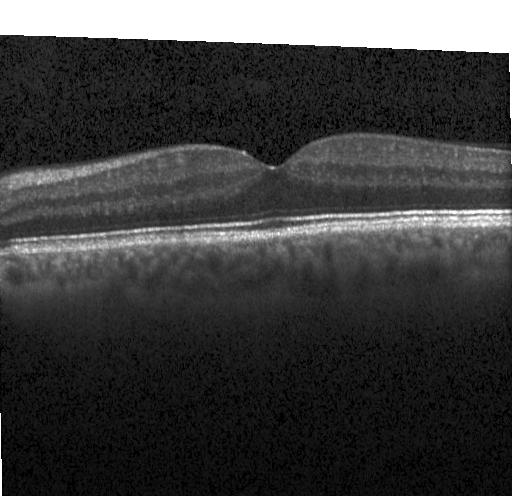
Horizontal scan through the fovea, Heidelberg Spectralis OCT system, retinal OCT cross-section — The scan shows neither choroidal neovascularization, diabetic macular edema, nor drusen.